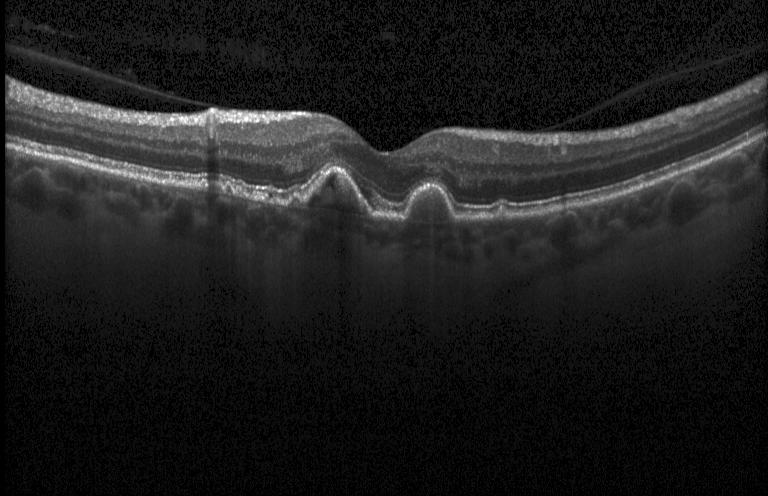

Diagnosis: drusen.